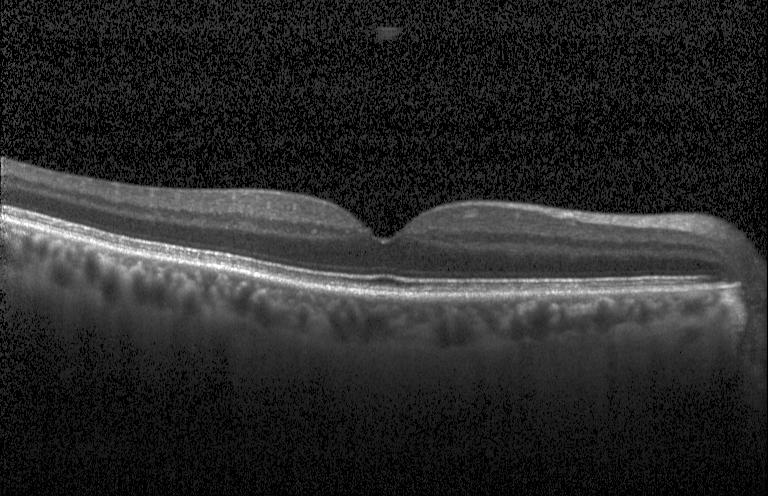
Optical coherence tomography B-scan — No choroidal neovascularization, no diabetic macular edema, and no drusen.